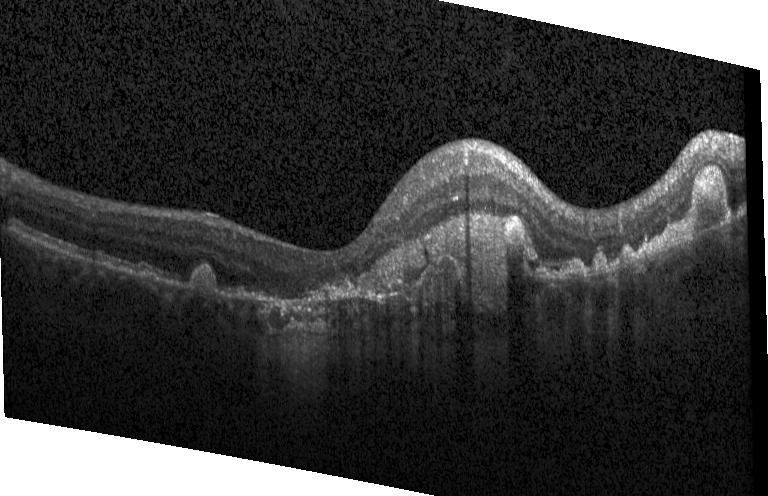 Centered on the fovea. Heidelberg Spectralis OCT system. Retinal OCT cross-section. SD-OCT — This B-scan demonstrates CNV.